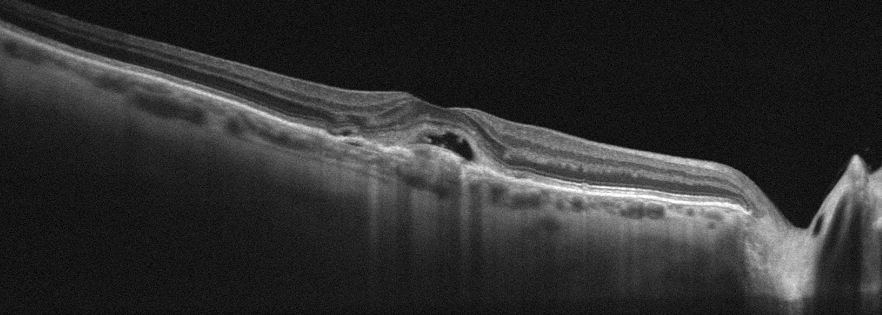 OD · optical coherence tomography B-scan · acquired on an Optovue Avanti RTVue XR · macular scan — The scan shows age-related macular degeneration (AMD).